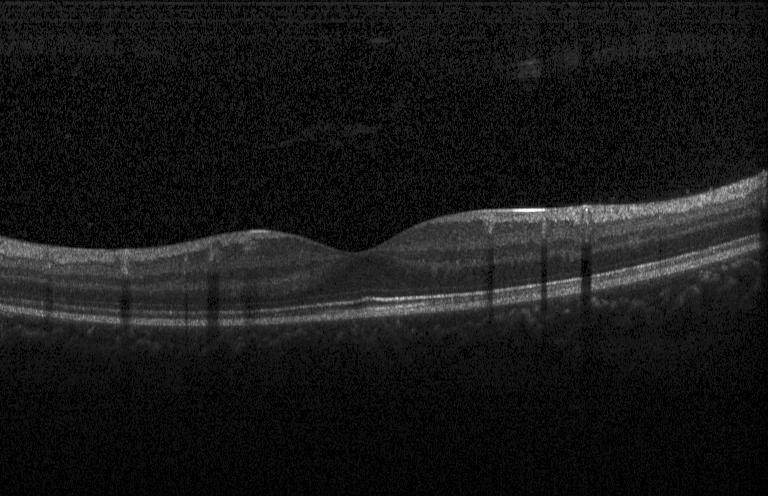
Horizontal scan through the fovea · acquired on a Heidelberg Spectralis · optical coherence tomography scan · spectral-domain OCT
Macular OCT: no CNV, DME, or drusen.